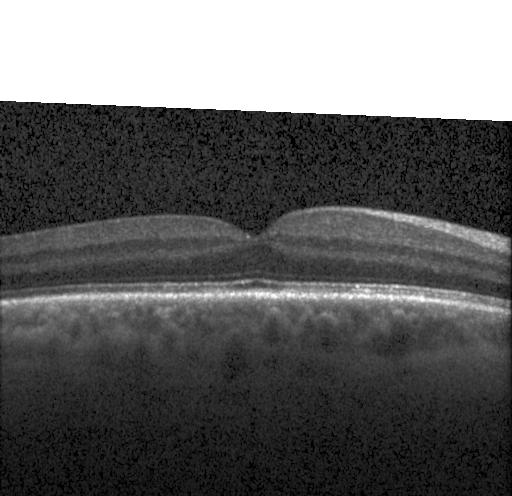

Optical coherence tomography B-scan · Heidelberg Spectralis OCT system — Finding: neither choroidal neovascularization, diabetic macular edema, nor drusen.